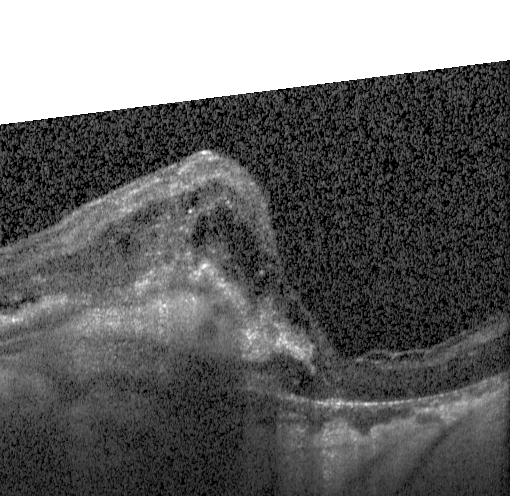

Optical coherence tomography B-scan — Impression: a choroidal neovascular membrane.